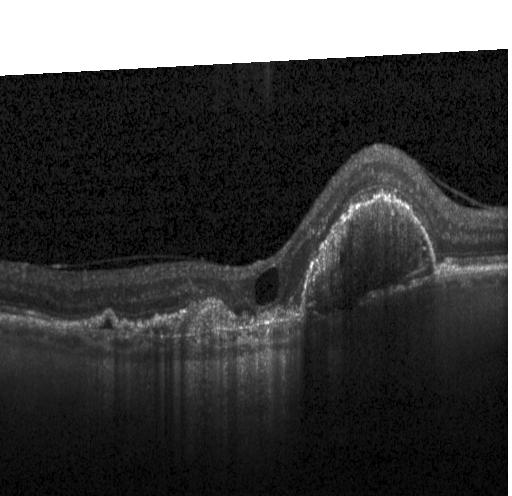

Impression: a choroidal neovascular membrane.